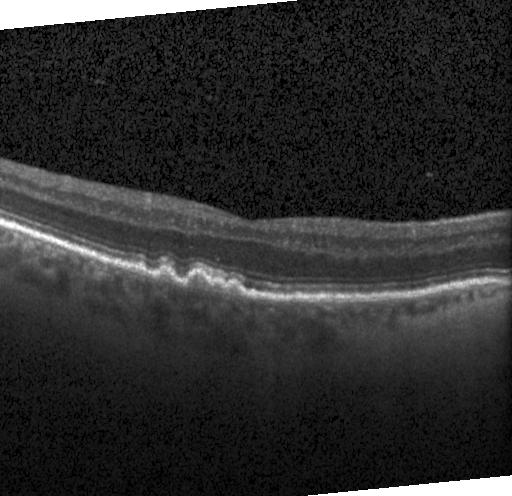 Retinal OCT cross-section showing sub-RPE drusenoid deposits.